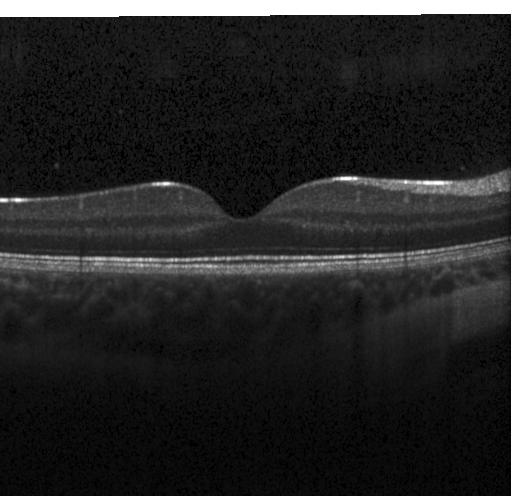

Through the macula, SD-OCT, retinal OCT B-scan.
Diagnosis: neither CNV, DME, nor drusen.